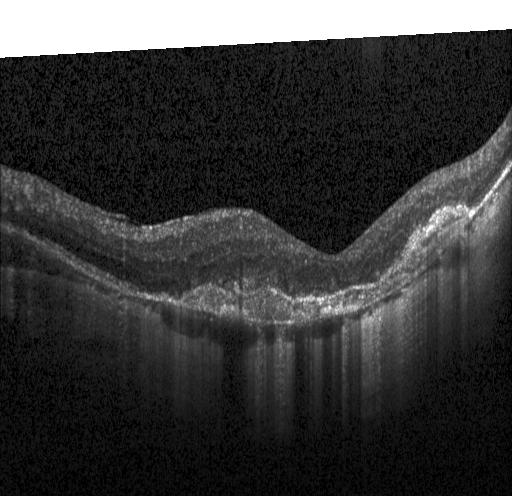
Optical coherence tomography scan
The scan shows a choroidal neovascular membrane.